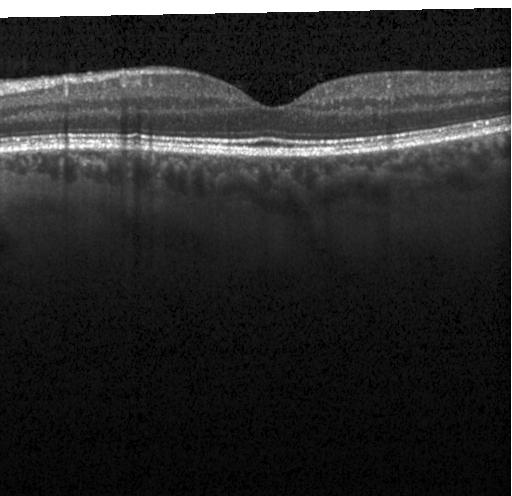
Assessment: no evidence of CNV, DME, or drusen.